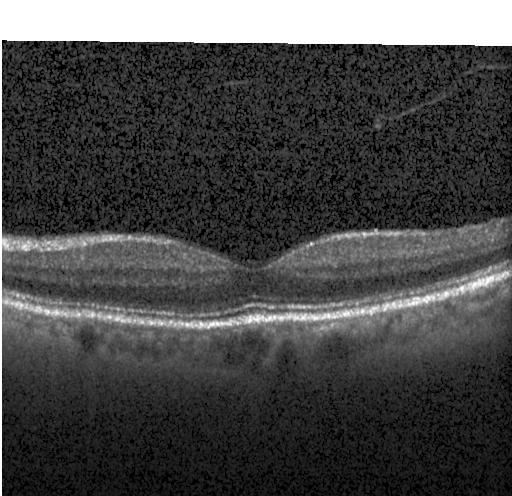

Acquired on a Heidelberg Spectralis · retinal OCT cross-section · centered on the fovea. The scan shows no choroidal neovascularization, no diabetic macular edema, and no drusen.